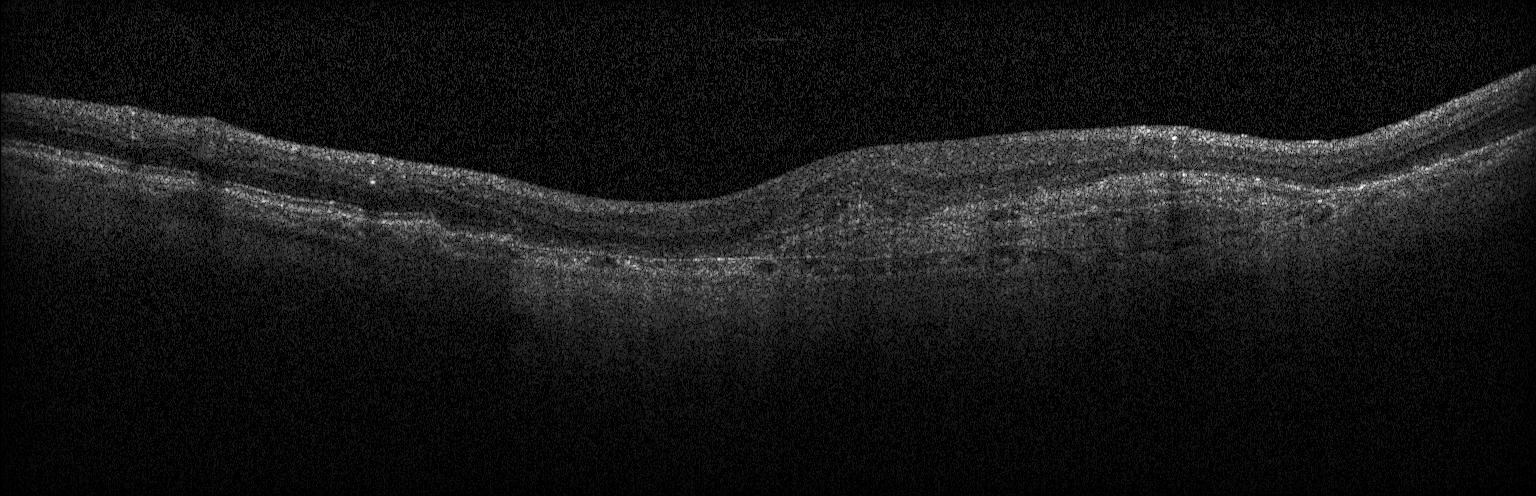
Heidelberg Spectralis OCT system, OCT line scan
Diagnosis: choroidal neovascularization (CNV).